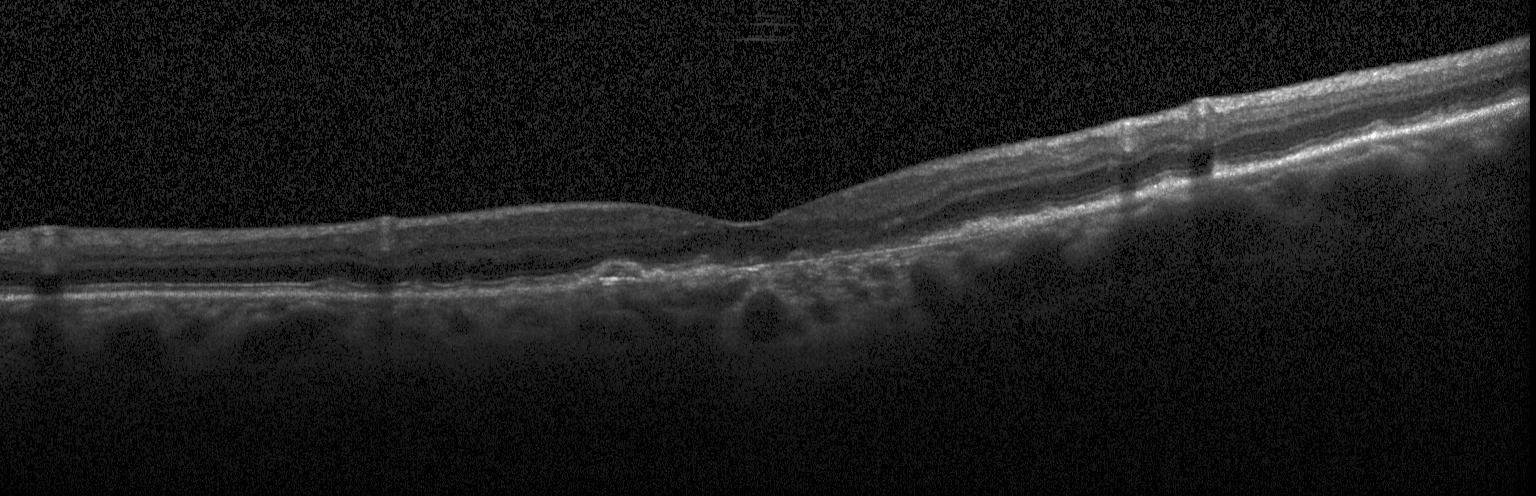

Optical coherence tomography scan, spectral-domain optical coherence tomography.
Assessment: CNV.